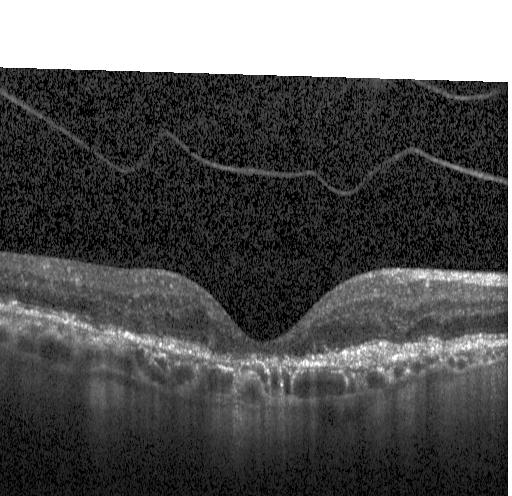 Impression: a choroidal neovascular membrane.